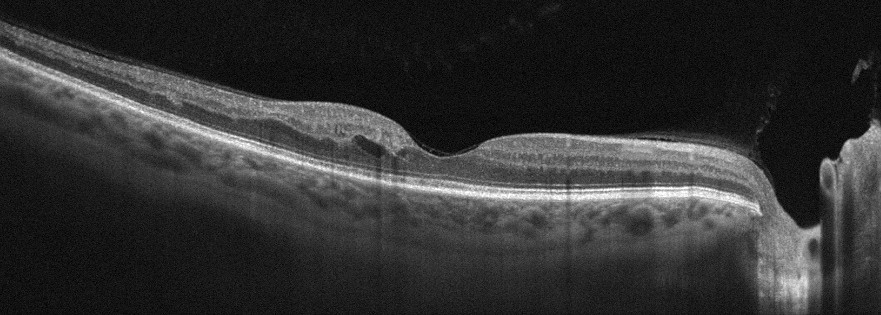
Macular OCT: DME.